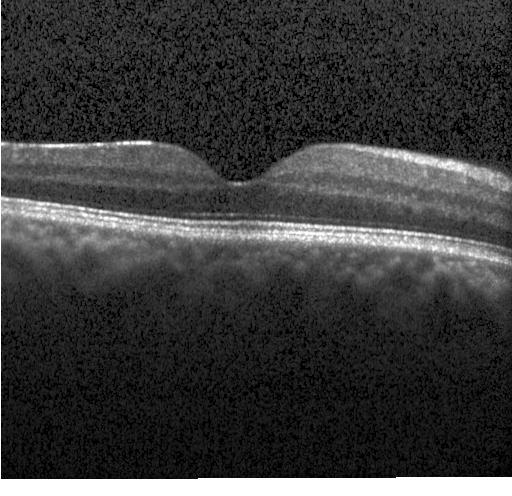

Retinal OCT B-scan. Centered on the fovea. Instrument: Heidelberg Spectralis. Spectral-domain OCT — Impression: no CNV, no DME, and no drusen.